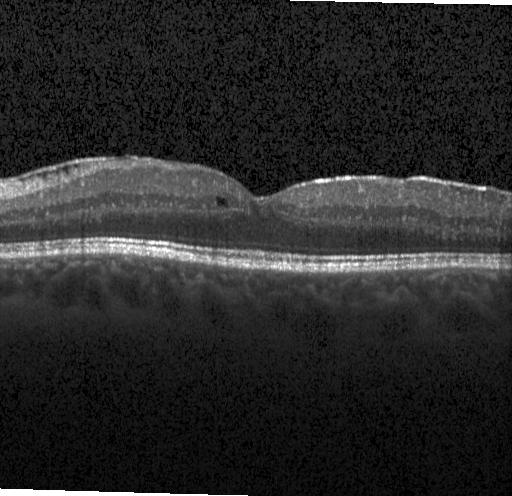
Acquired on a Heidelberg Spectralis. Optical coherence tomography scan. Spectral-domain optical coherence tomography. Fovea-centered — Macular OCT: DME.